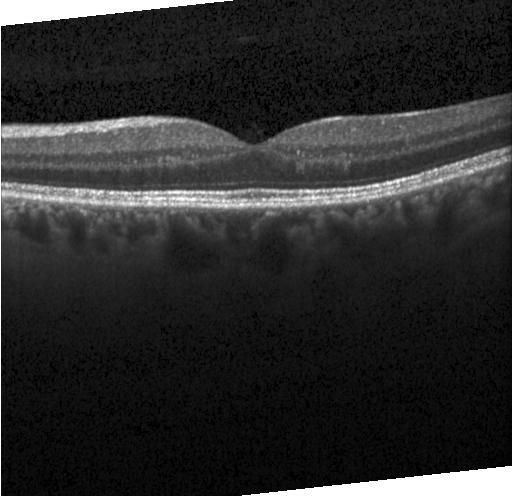 OCT B-scan. Neither choroidal neovascularization, diabetic macular edema, nor drusen.